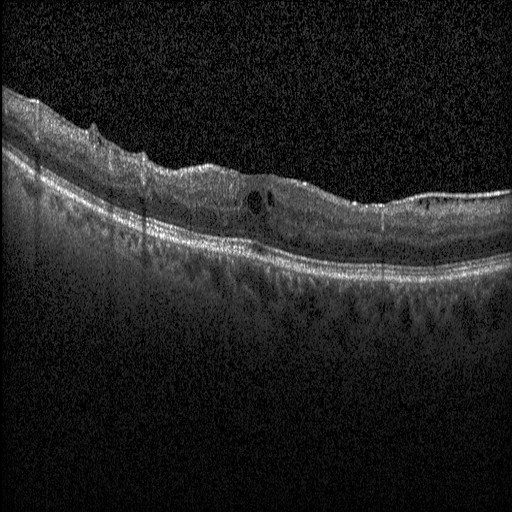 Instrument: Heidelberg Spectralis; centered on the fovea; OCT B-scan
The scan shows DME.